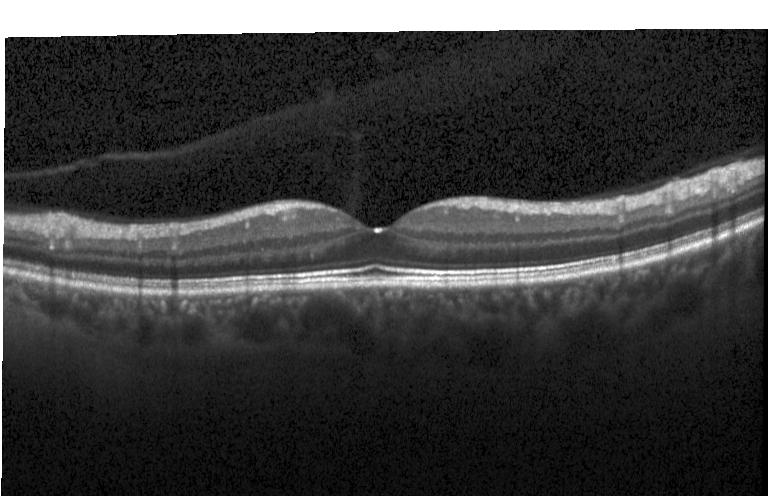

Spectral-domain optical coherence tomography; macular scan; Heidelberg Spectralis OCT system; retinal OCT B-scan.
OCT finding: no evidence of choroidal neovascularization, diabetic macular edema, or drusen.